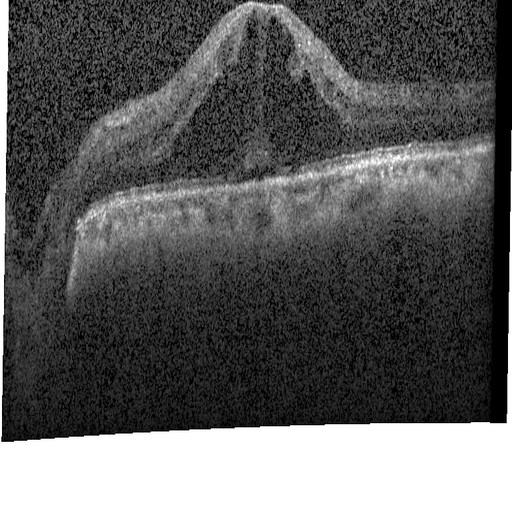 OCT B-scan. Finding: diabetic macular edema (DME).